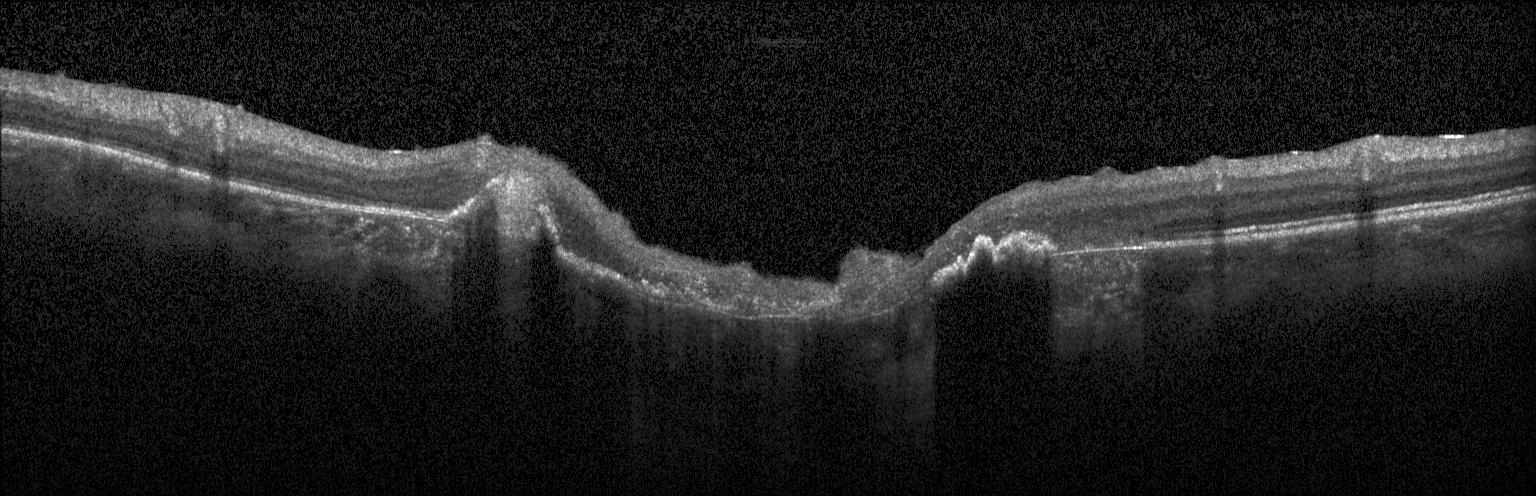
OCT finding: choroidal neovascularization (CNV).